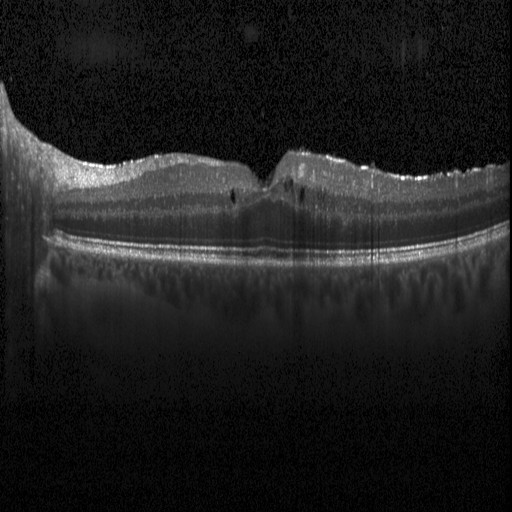
Optical coherence tomography scan; spectral-domain optical coherence tomography; instrument: Heidelberg Spectralis — Diagnosis: diabetic macular edema.